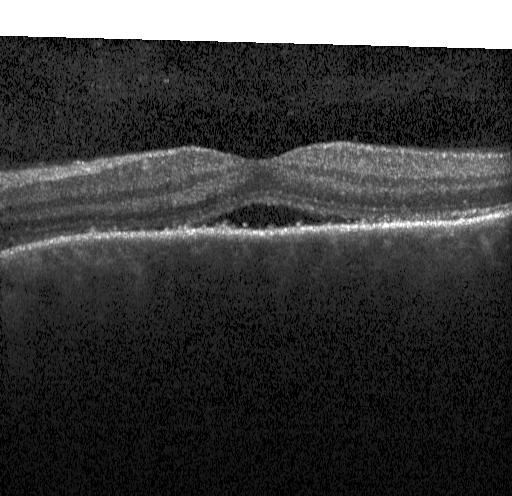
OCT scan showing choroidal neovascularization.